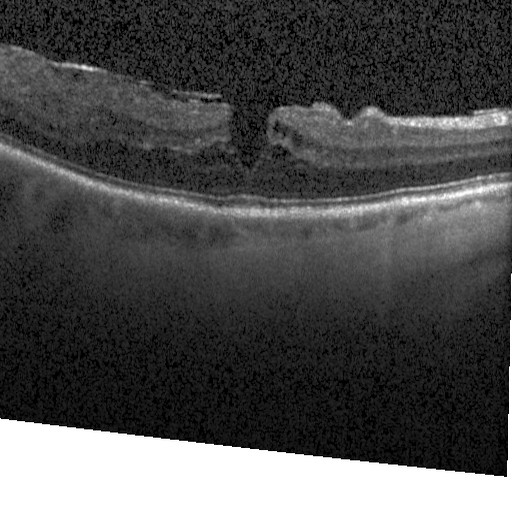
OCT B-scan
Dx: diabetic macular edema (DME).